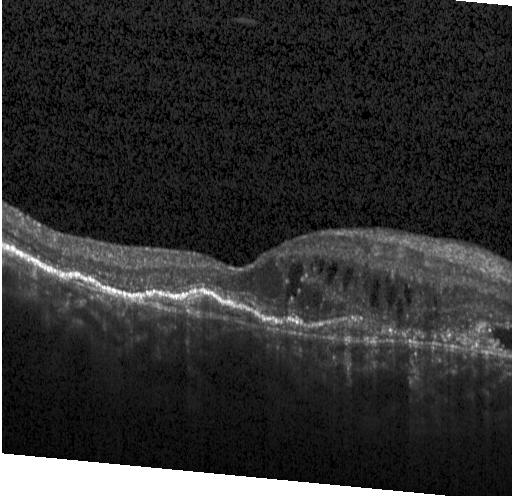 Horizontal scan through the fovea · retinal OCT B-scan · instrument: Heidelberg Spectralis.
Macular OCT: a choroidal neovascular membrane.